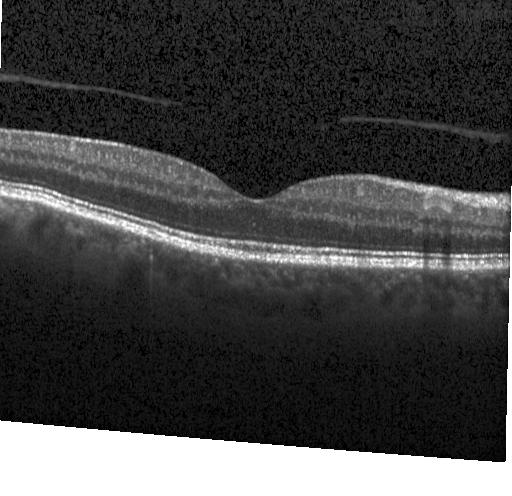 Impression: no evidence of choroidal neovascularization, diabetic macular edema, or drusen.